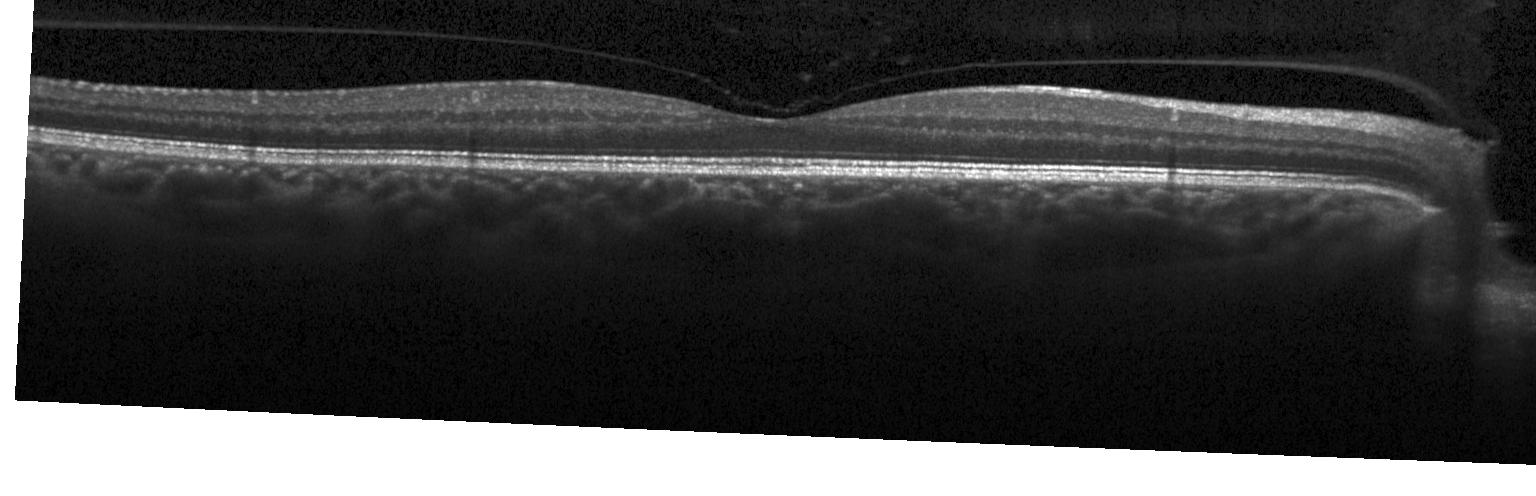

SD-OCT. Acquired on a Heidelberg Spectralis. Optical coherence tomography B-scan. Centered on the fovea — This B-scan demonstrates no choroidal neovascularization, no diabetic macular edema, and no drusen.